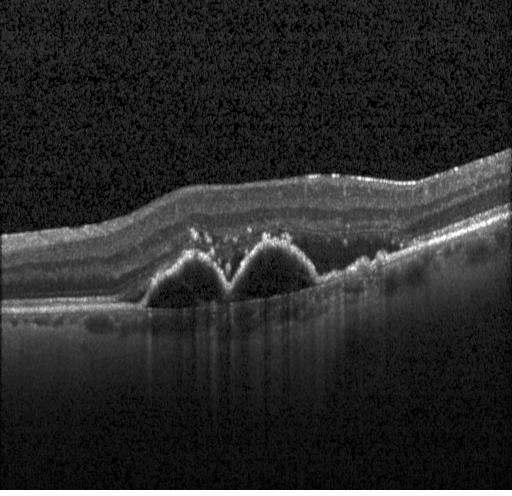 OCT B-scan showing a choroidal neovascular membrane.